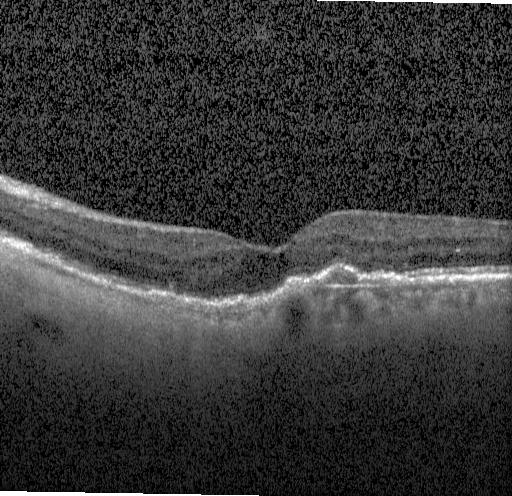

OCT line scan · through the macula. Diagnosis: a choroidal neovascular membrane.